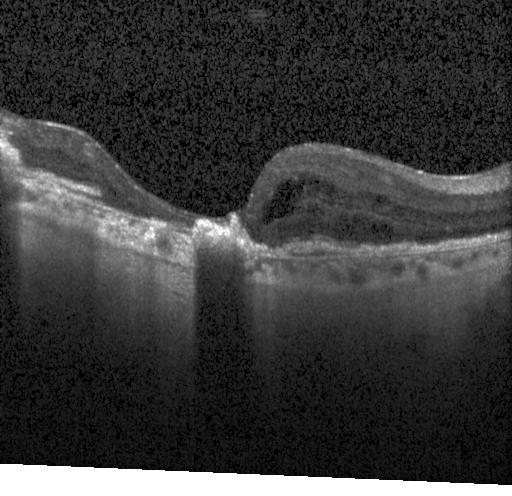

Optical coherence tomography B-scan, fovea-centered.
The scan shows a choroidal neovascular membrane.